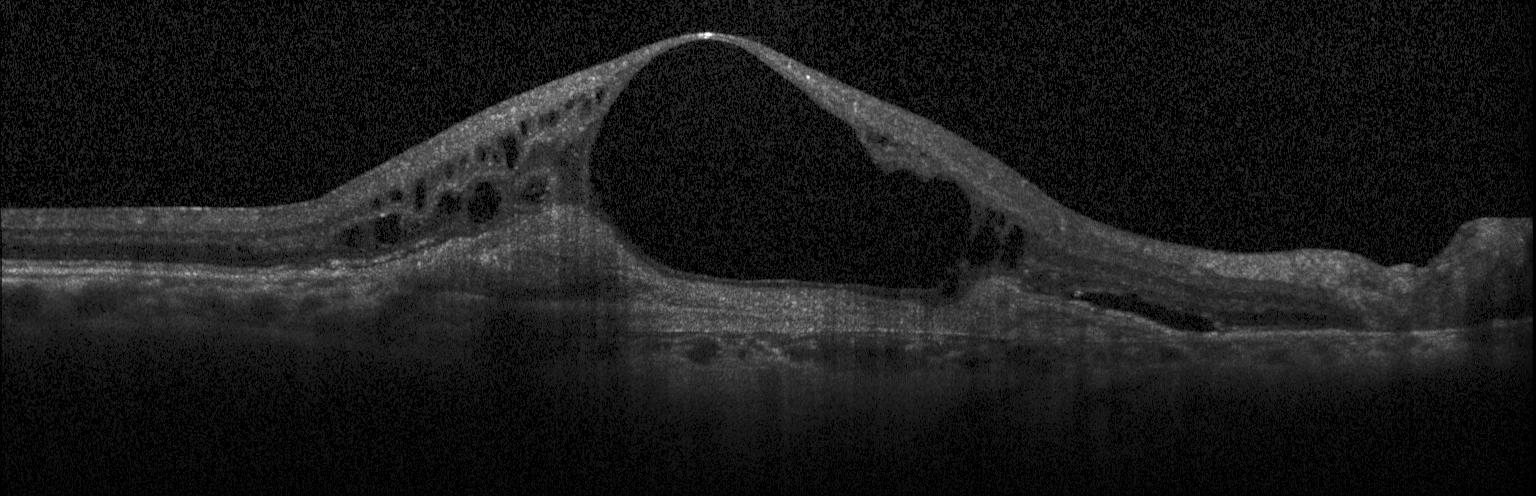
OCT line scan; Heidelberg Spectralis — Finding: a choroidal neovascular membrane.